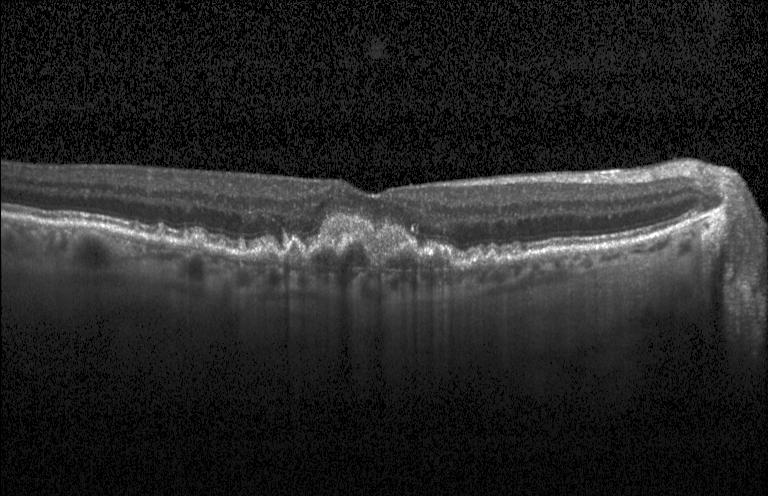

Spectral-domain OCT · centered on the fovea · retinal OCT B-scan · Heidelberg Spectralis OCT system.
Diagnosis: choroidal neovascularization.